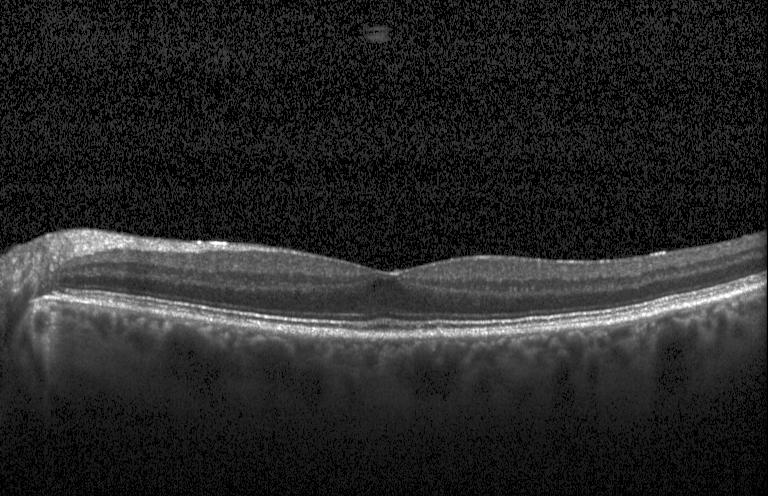 Assessment: no choroidal neovascularization, no diabetic macular edema, and no drusen.